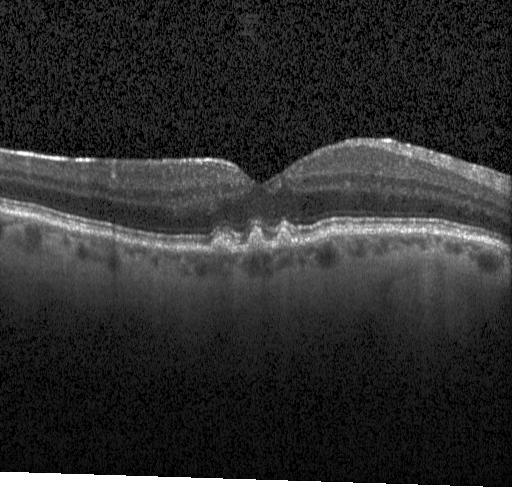
Spectral-domain optical coherence tomography; retinal OCT cross-section.
Finding: sub-RPE drusenoid deposits.